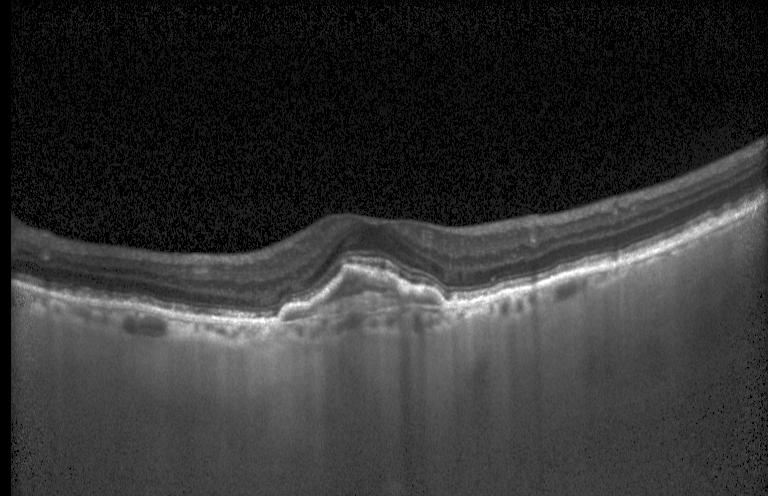 Impression: choroidal neovascularization.